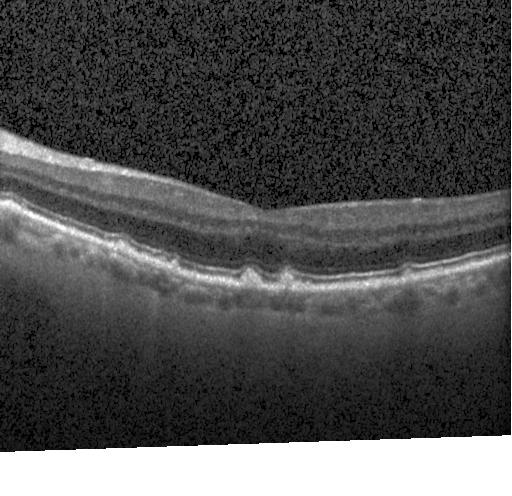
OCT line scan; Heidelberg Spectralis OCT system; centered on the fovea. Impression: multiple drusen.